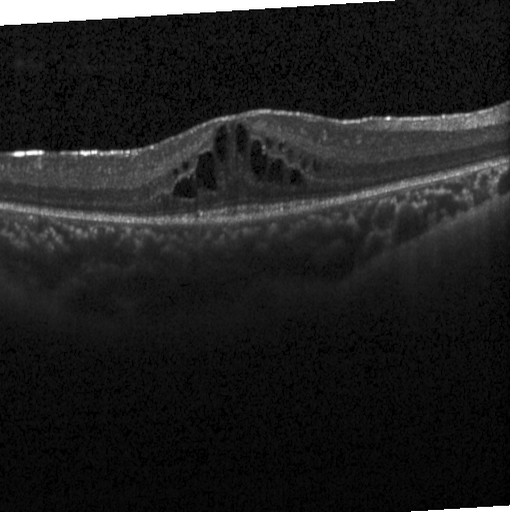

Spectral-domain OCT B-scan: DME.